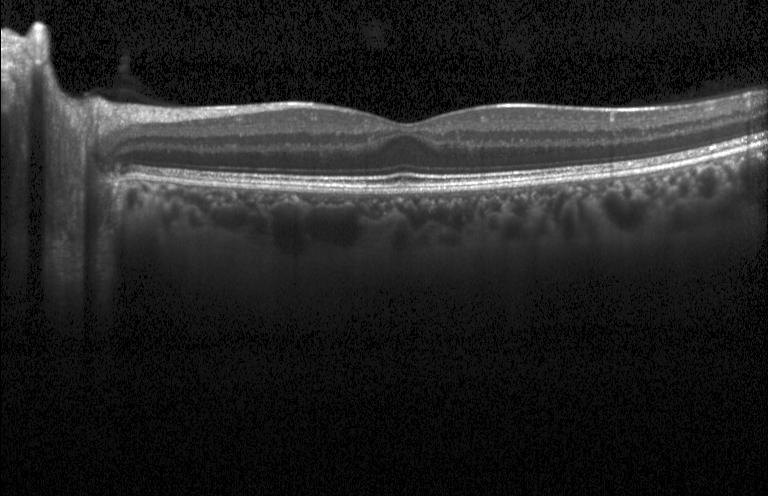
Diagnosis: no evidence of CNV, DME, or drusen.